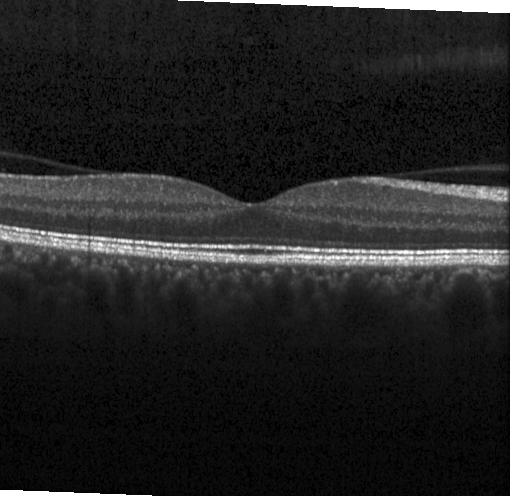 Through the macula, retinal OCT cross-section, SD-OCT.
Diagnosis: neither CNV, DME, nor drusen.